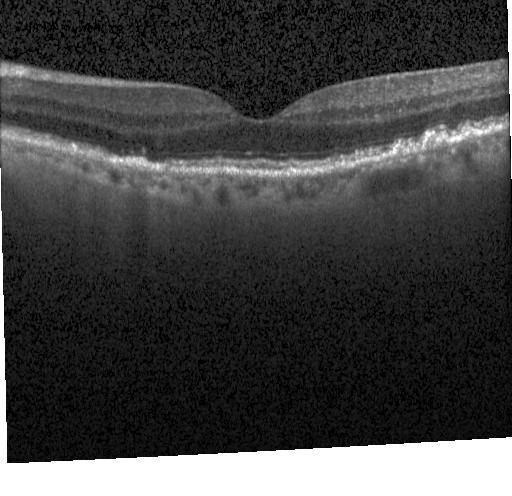

Retinal OCT B-scan; Heidelberg Spectralis. The scan shows sub-RPE drusenoid deposits.